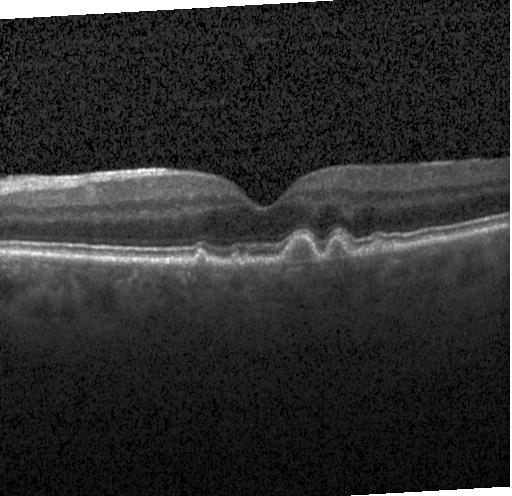

Optical coherence tomography scan, spectral-domain OCT, Heidelberg Spectralis. Macular OCT: drusen.